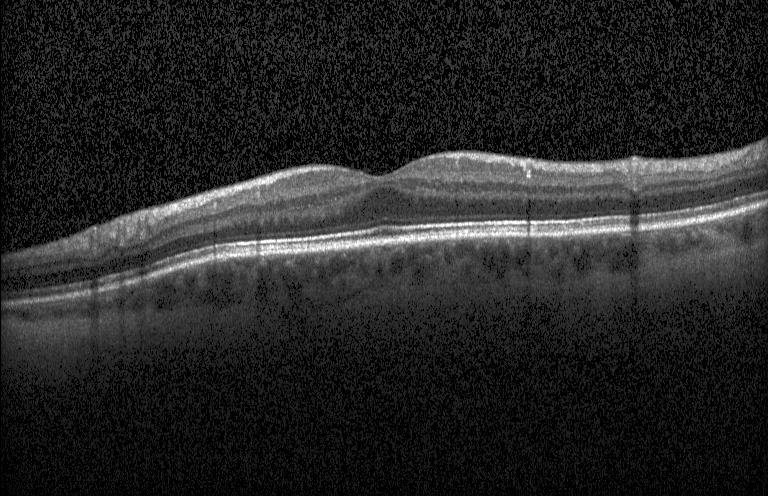

No choroidal neovascularization, no diabetic macular edema, and no drusen.